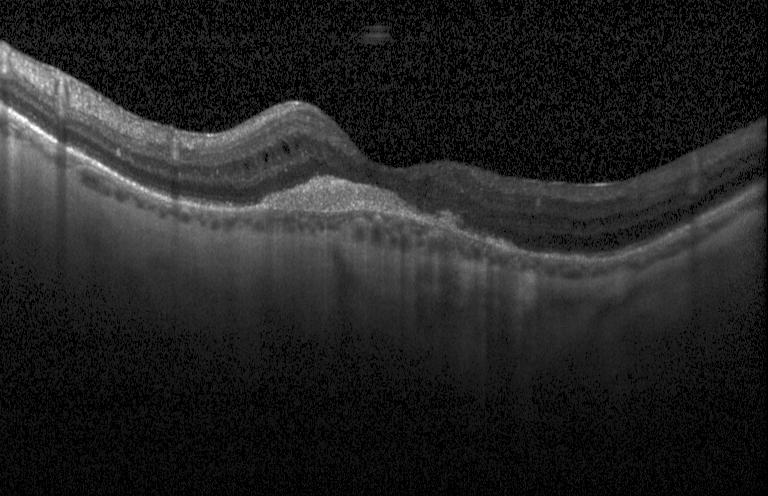
Finding: choroidal neovascularization.